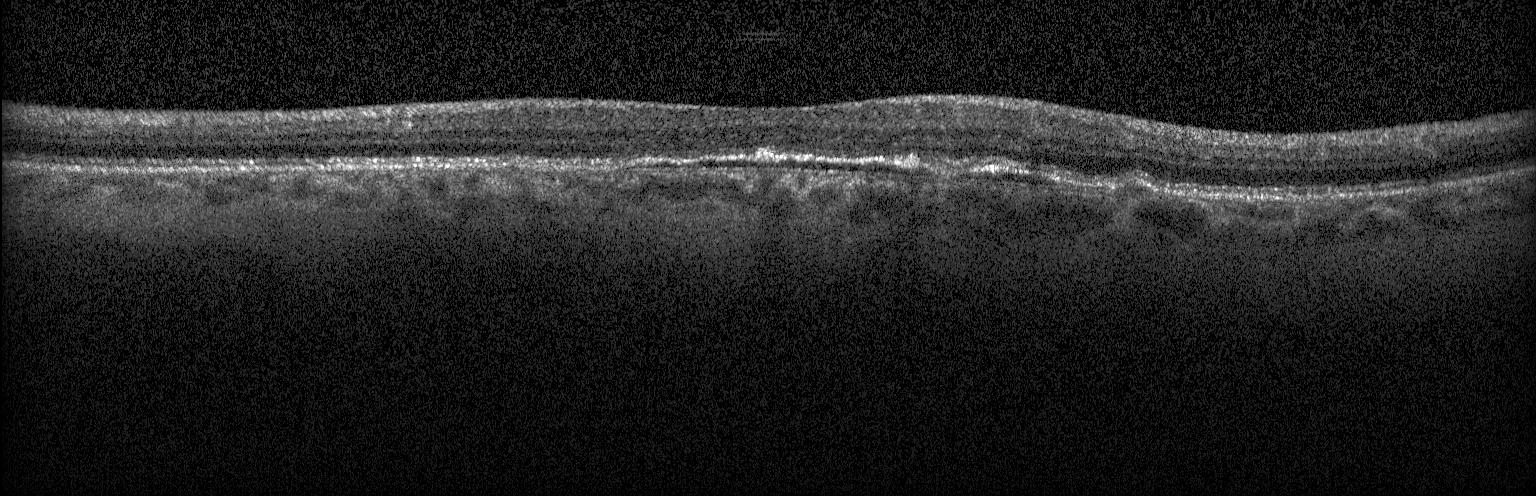 OCT line scan — Impression: choroidal neovascularization.